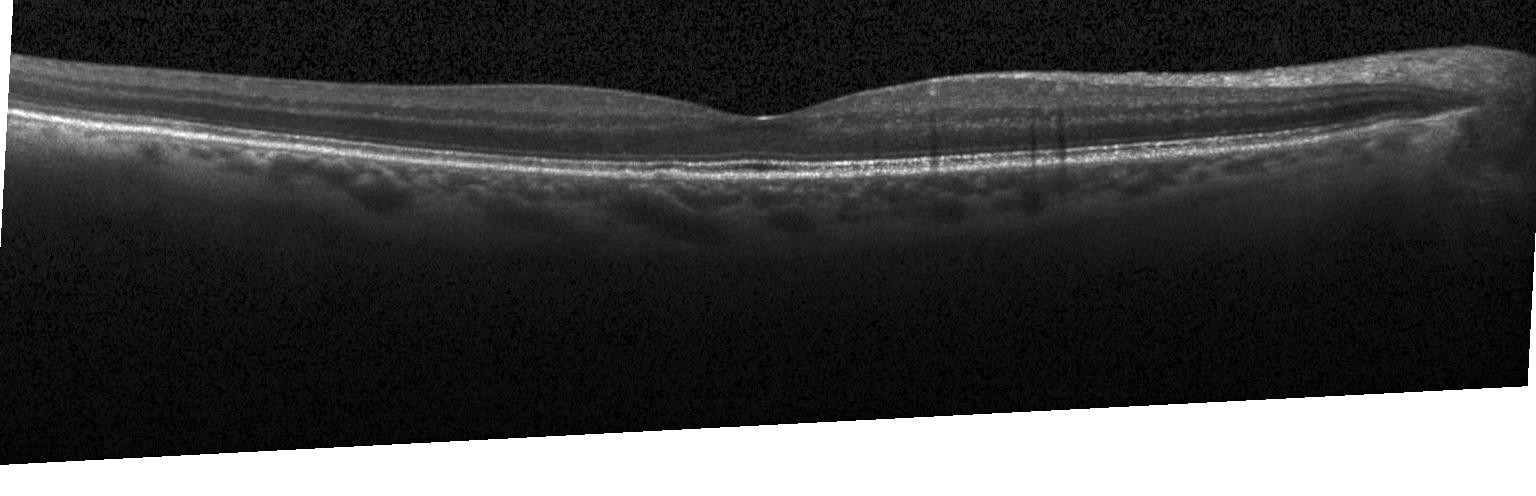

OCT B-scan.
Macular OCT: no choroidal neovascularization, diabetic macular edema, or drusen.